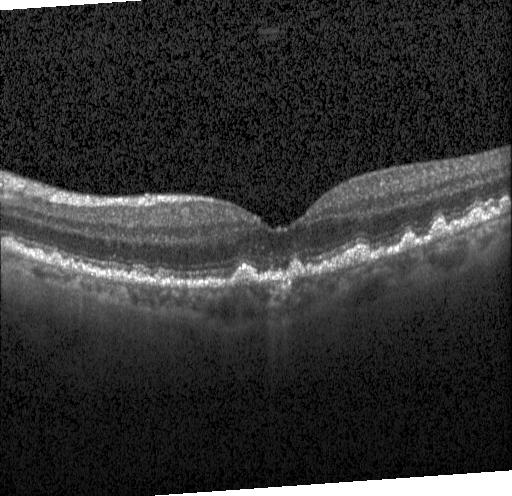
Retinal OCT B-scan; spectral-domain optical coherence tomography.
The scan shows sub-RPE drusenoid deposits.